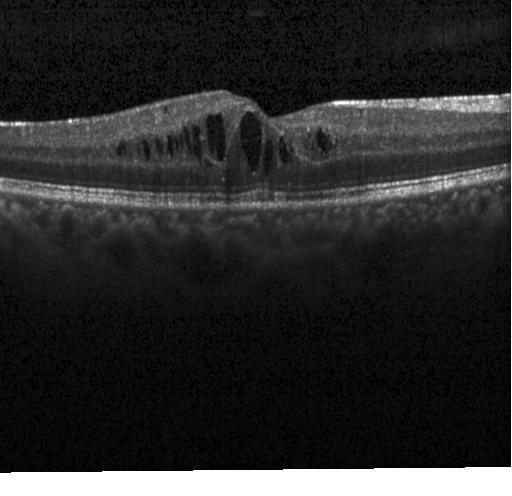 Impression: diabetic macular edema.